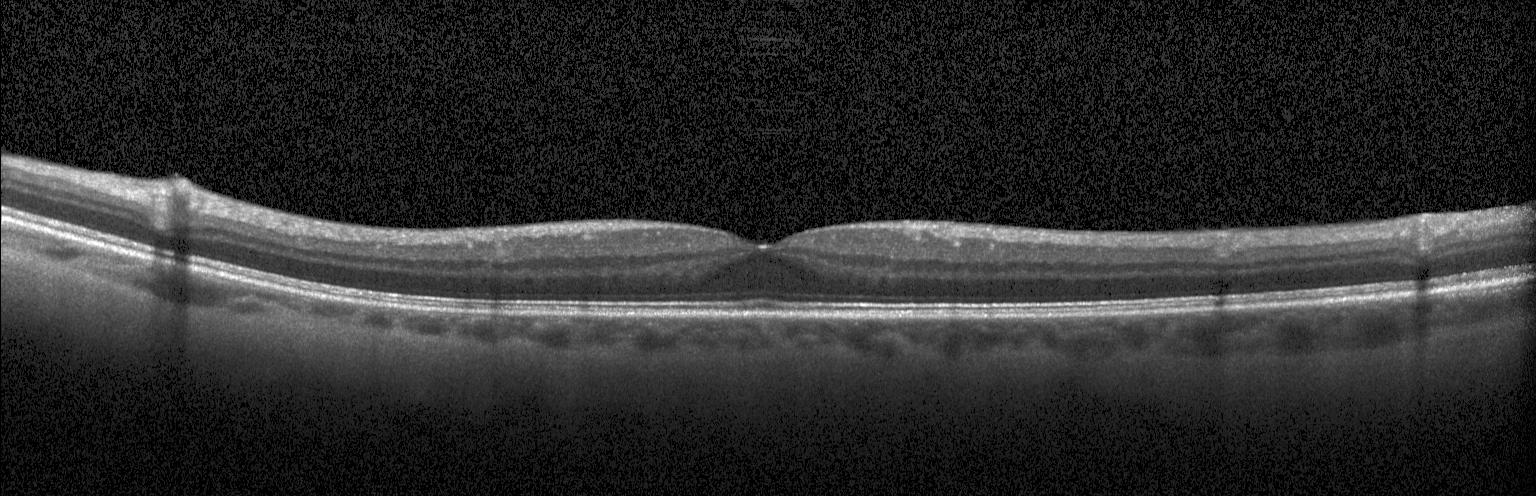

Spectral-domain OCT; macular scan; OCT line scan. Diagnosis: no choroidal neovascularization, diabetic macular edema, or drusen.